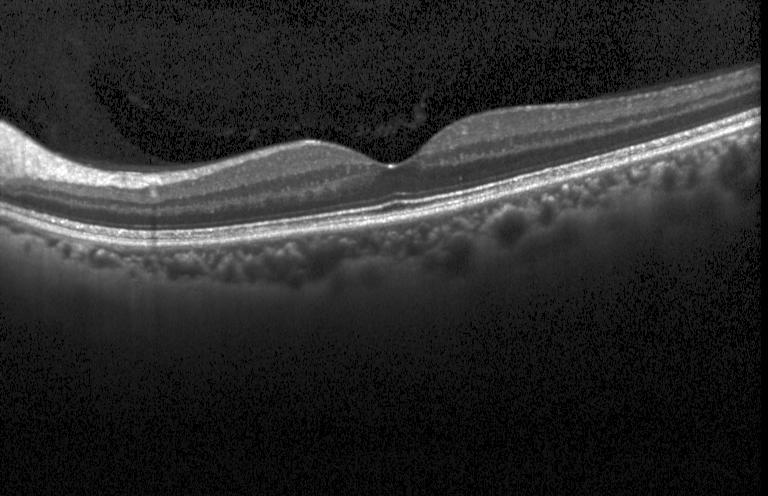
OCT line scan; Heidelberg Spectralis OCT system; horizontal scan through the fovea; spectral-domain OCT
This B-scan demonstrates neither CNV, DME, nor drusen.